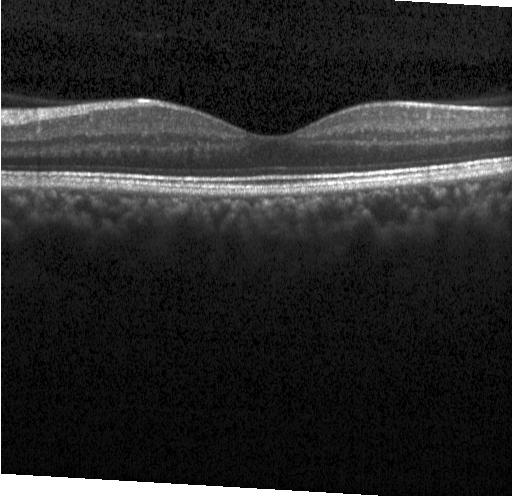

OCT finding: neither choroidal neovascularization, diabetic macular edema, nor drusen.